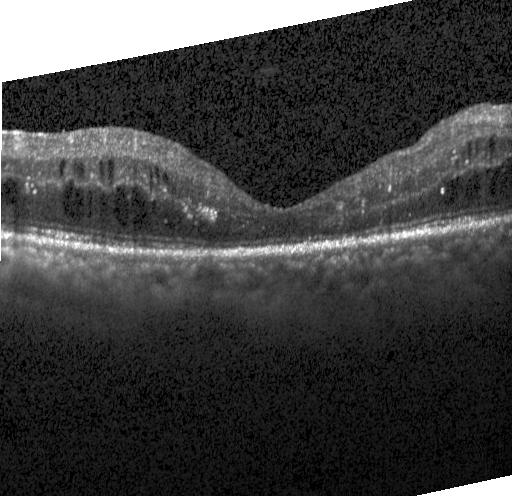

Heidelberg Spectralis OCT system · retinal OCT cross-section. Finding: diabetic macular edema.